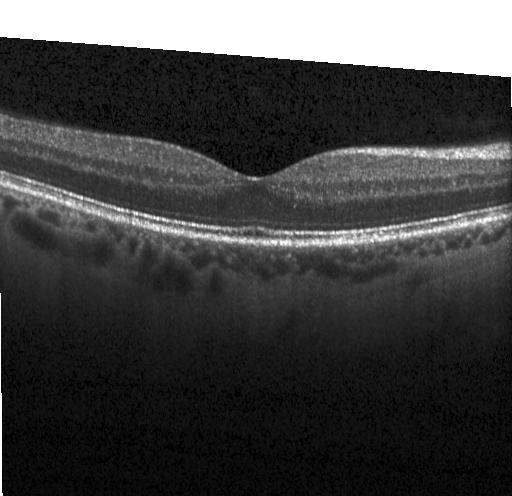
Macular OCT demonstrating neither choroidal neovascularization, diabetic macular edema, nor drusen.